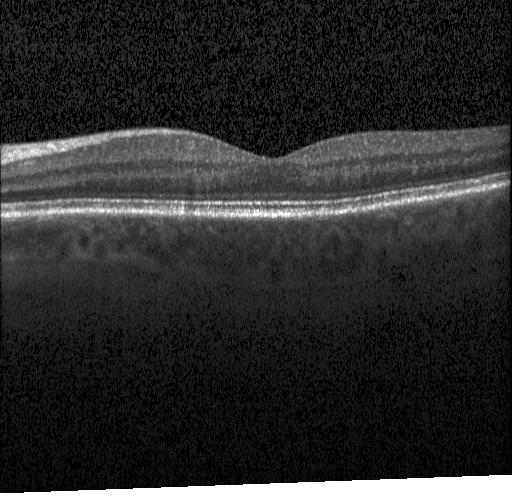
Macular OCT demonstrating no CNV, no DME, and no drusen.